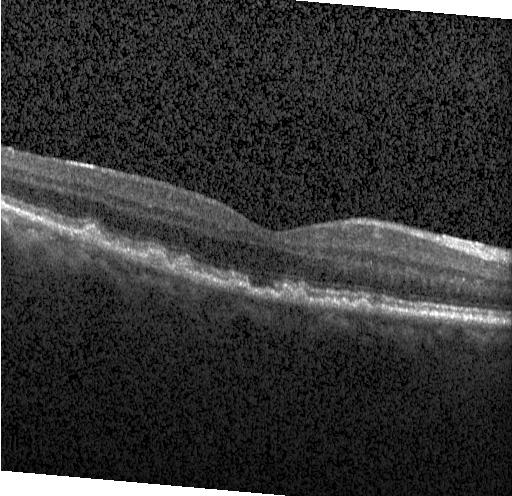

Macular OCT: multiple drusen.